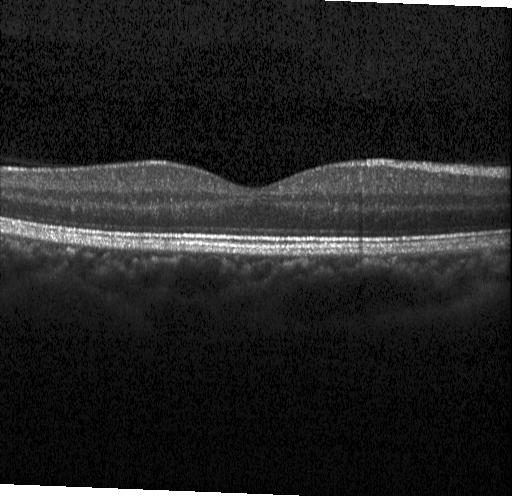

Horizontal scan through the fovea · OCT line scan — Diagnosis: no choroidal neovascularization, no diabetic macular edema, and no drusen.